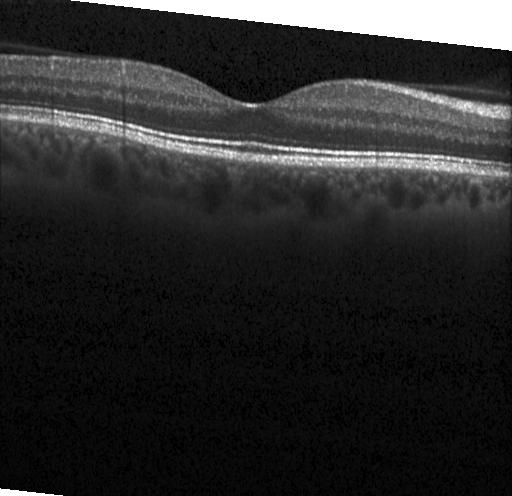 Optical coherence tomography scan — Diagnosis: no choroidal neovascularization, diabetic macular edema, or drusen.